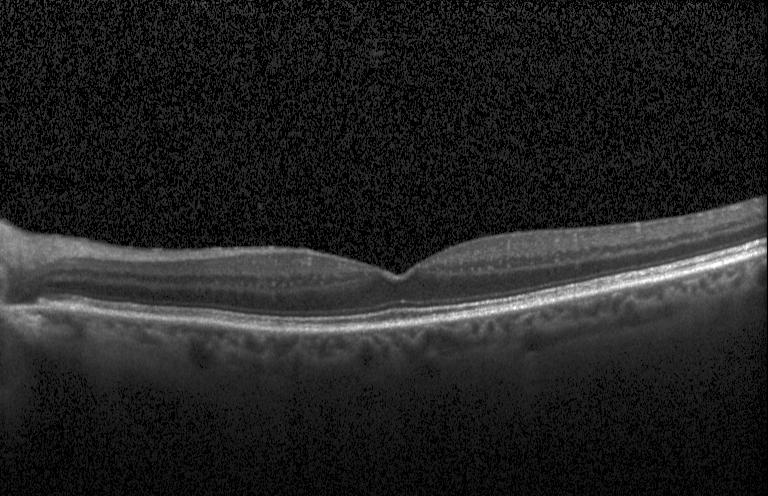 Retinal OCT B-scan — Neither choroidal neovascularization, diabetic macular edema, nor drusen.